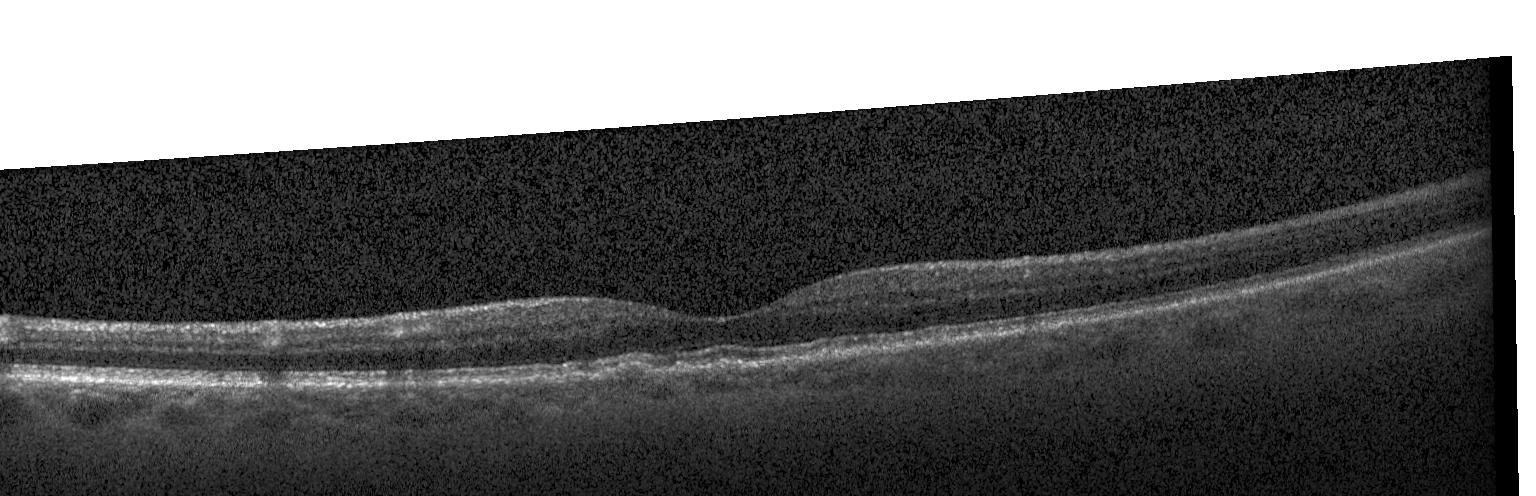

OCT B-scan. Impression: sub-RPE drusenoid deposits.